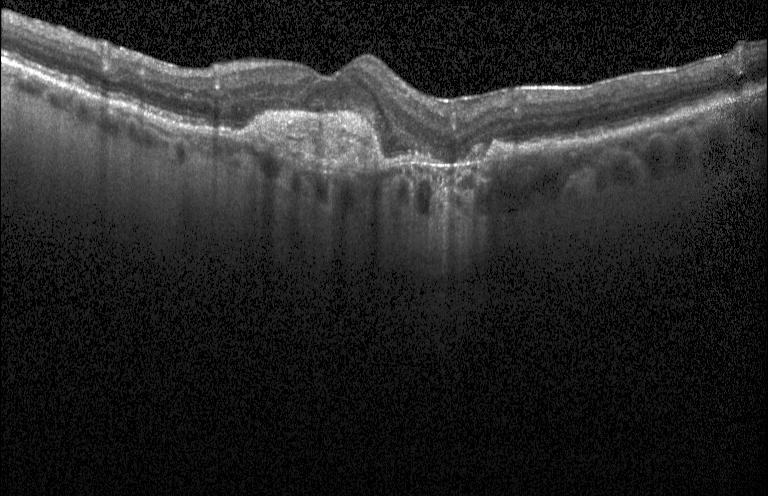

OCT finding: choroidal neovascularization.